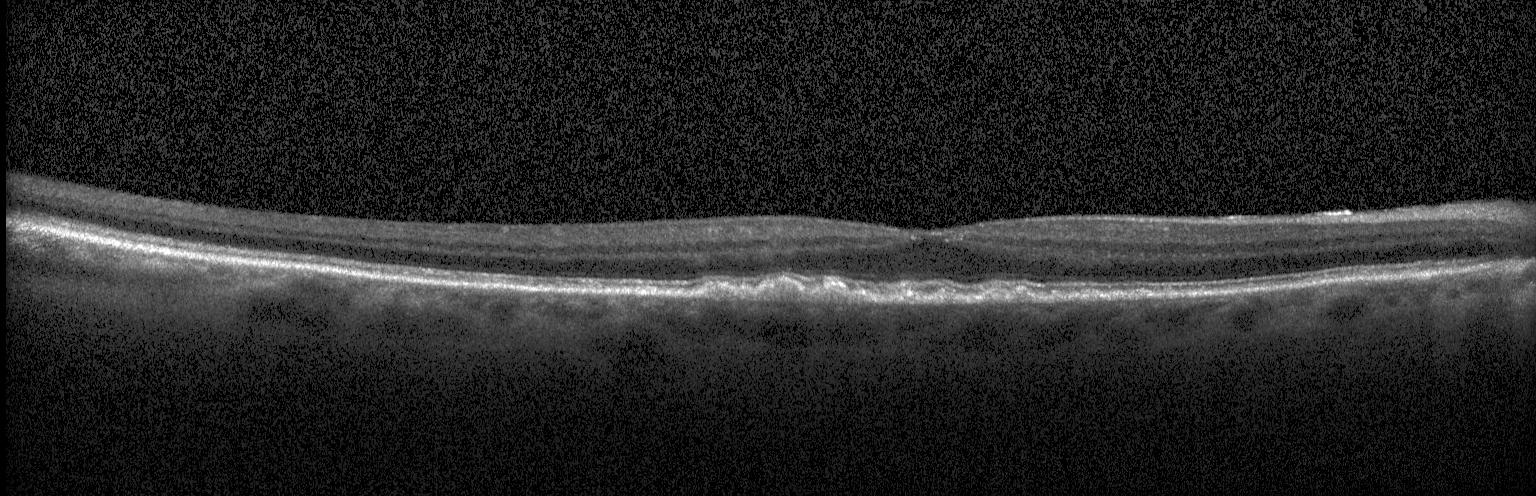 Spectral-domain OCT B-scan: drusen.